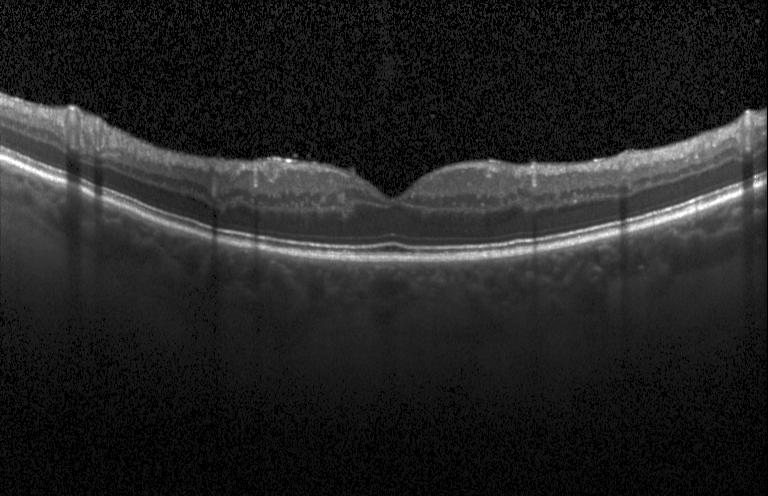
OCT B-scan showing no evidence of choroidal neovascularization, diabetic macular edema, or drusen.